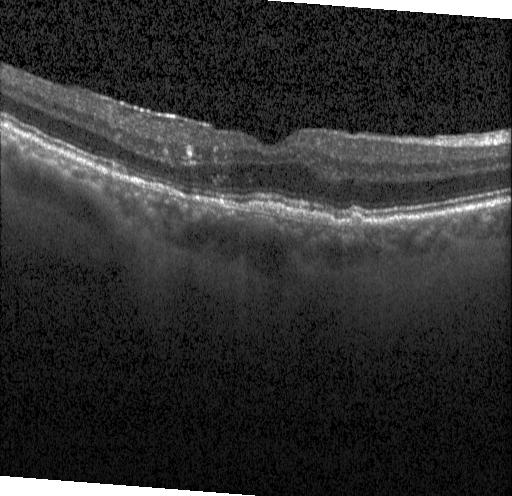

A choroidal neovascular membrane.